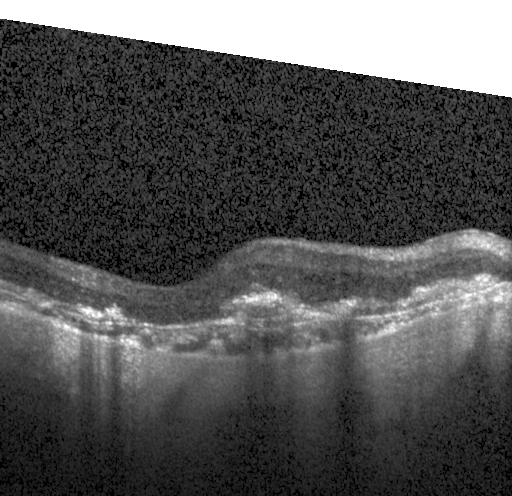 OCT line scan, SD-OCT, fovea-centered
Macular OCT: a choroidal neovascular membrane.